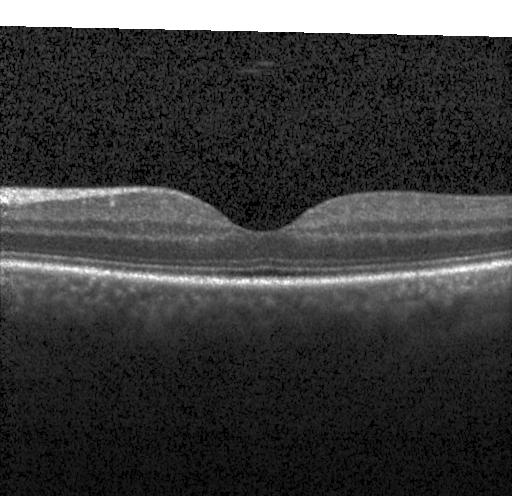 Diagnosis: no choroidal neovascularization, diabetic macular edema, or drusen.